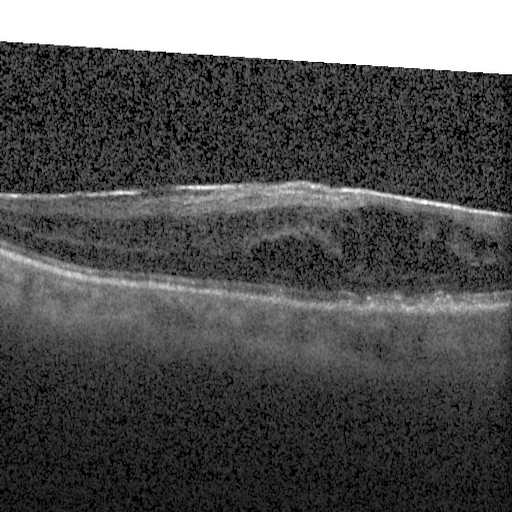
Optical coherence tomography scan. Spectral-domain OCT. Instrument: Heidelberg Spectralis. Fovea-centered.
This B-scan demonstrates diabetic macular edema.